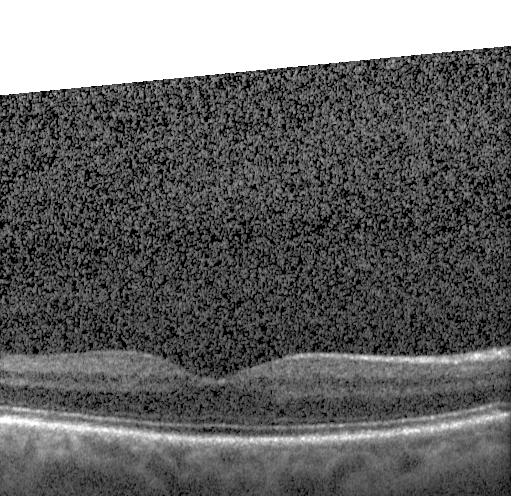
OCT line scan · horizontal scan through the fovea
Assessment: no evidence of choroidal neovascularization, diabetic macular edema, or drusen.